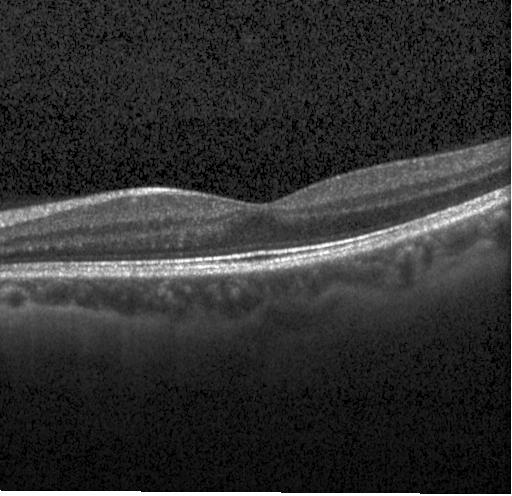 Macular OCT demonstrating no choroidal neovascularization, diabetic macular edema, or drusen.